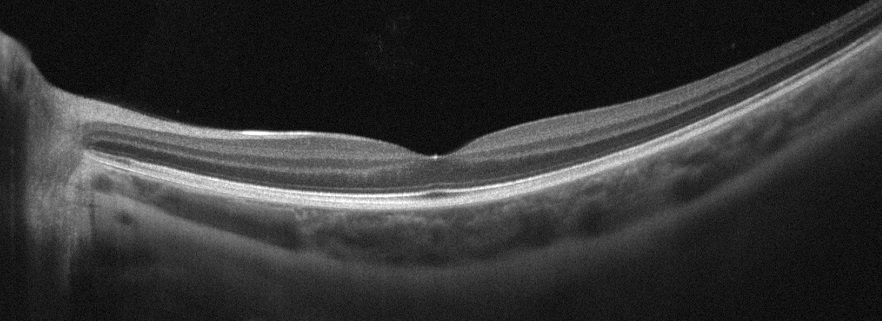
OCT scan showing no AMD, DME, ERM, RAO, RVO, or VID.